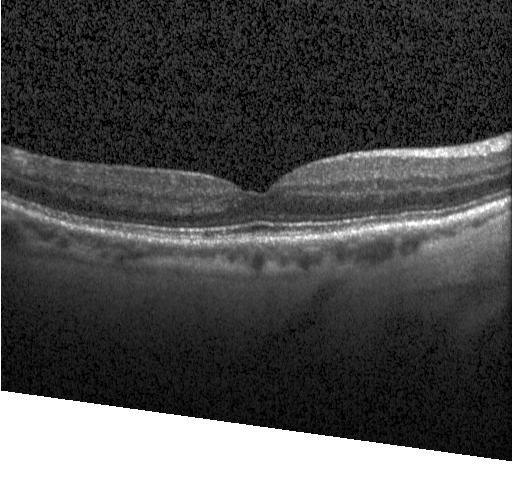

Spectral-domain optical coherence tomography · OCT B-scan · Heidelberg Spectralis. Finding: no evidence of CNV, DME, or drusen.